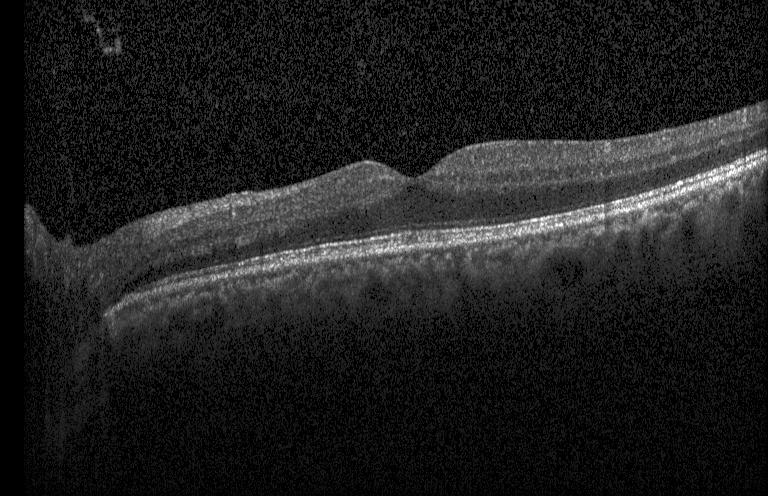
Finding: no choroidal neovascularization, diabetic macular edema, or drusen.